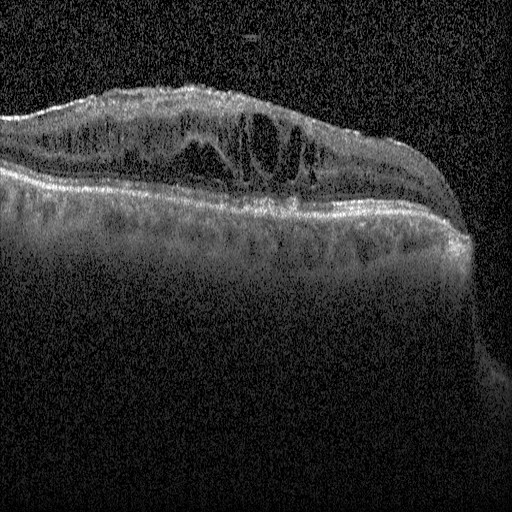

Acquired on a Heidelberg Spectralis. Retinal OCT cross-section
Macular OCT: diabetic macular edema (DME).